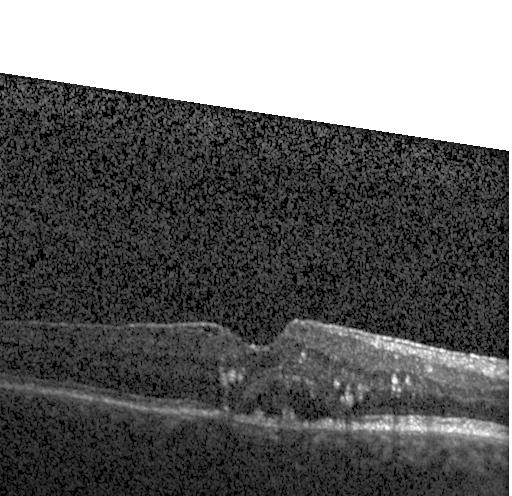

Retinal OCT cross-section showing CNV.